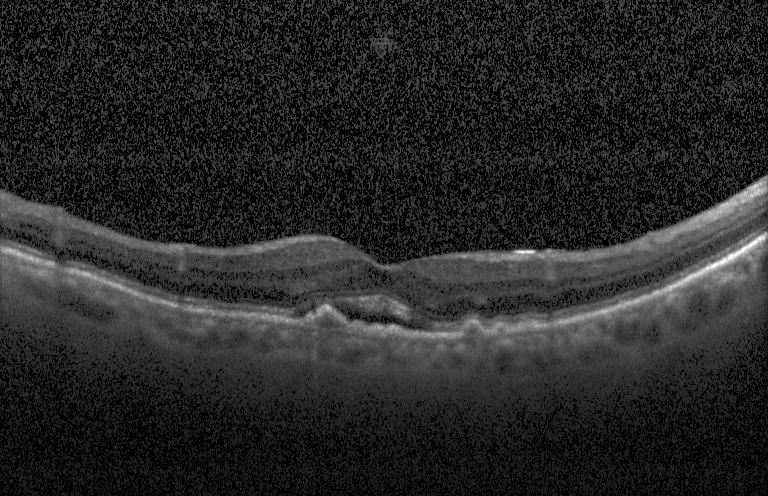 Retinal OCT B-scan · spectral-domain OCT · through the macula · Heidelberg Spectralis
Impression: choroidal neovascularization (CNV).